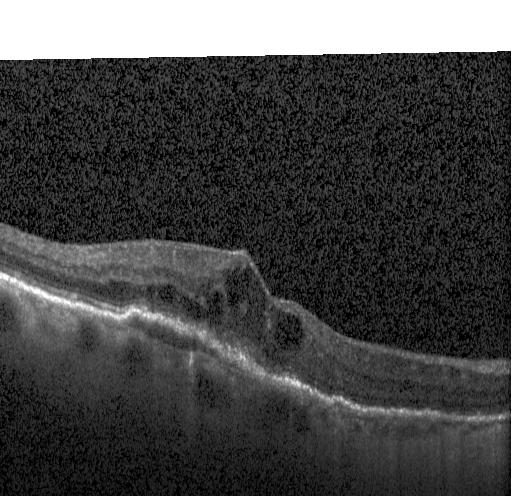
Finding: choroidal neovascularization (CNV).